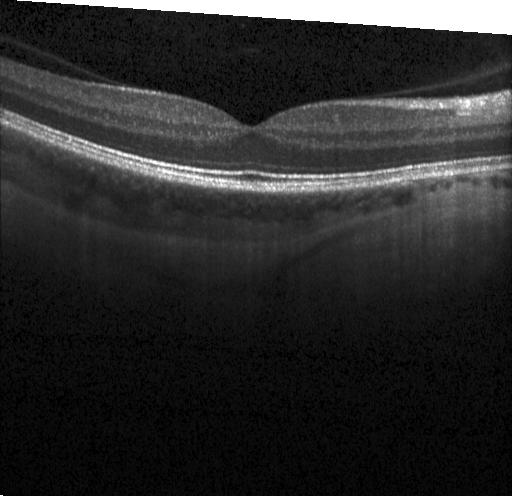 Impression: neither choroidal neovascularization, diabetic macular edema, nor drusen.